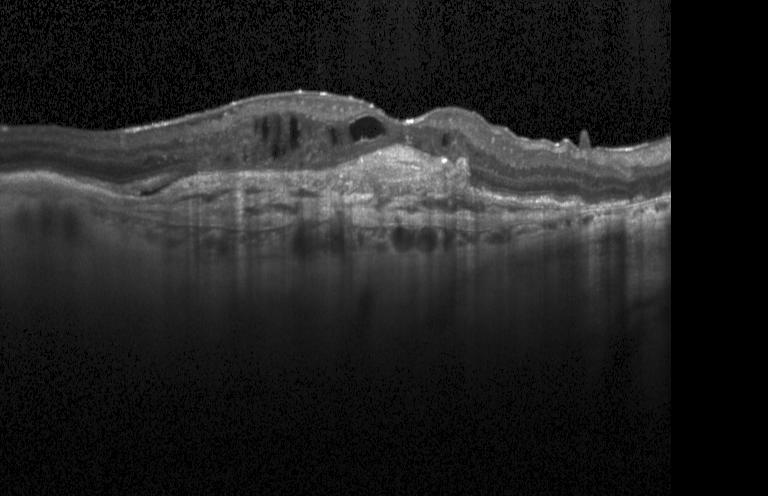

Retinal OCT cross-section.
This B-scan demonstrates CNV.